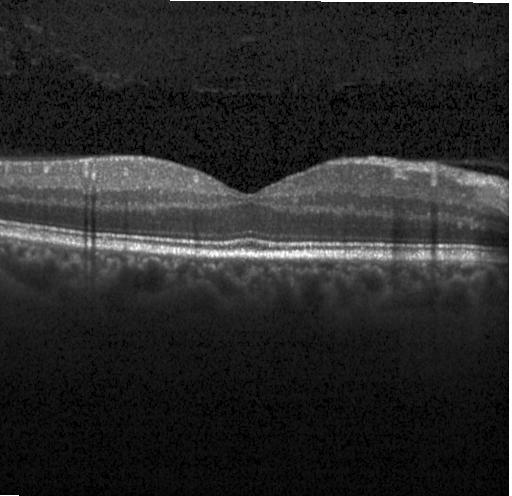

Retinal OCT B-scan. No choroidal neovascularization, no diabetic macular edema, and no drusen.